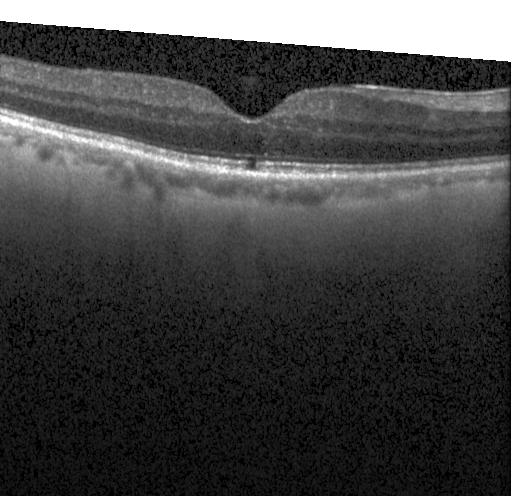

OCT B-scan. Diagnosis: no choroidal neovascularization, diabetic macular edema, or drusen.